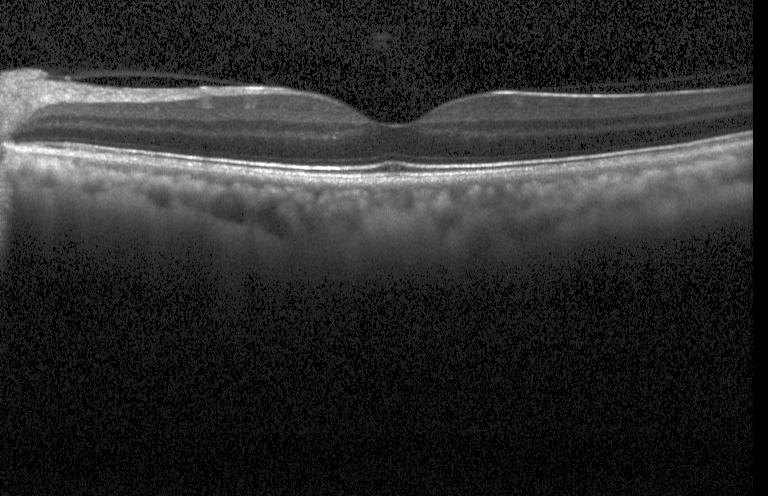 Dx: no CNV, DME, or drusen.